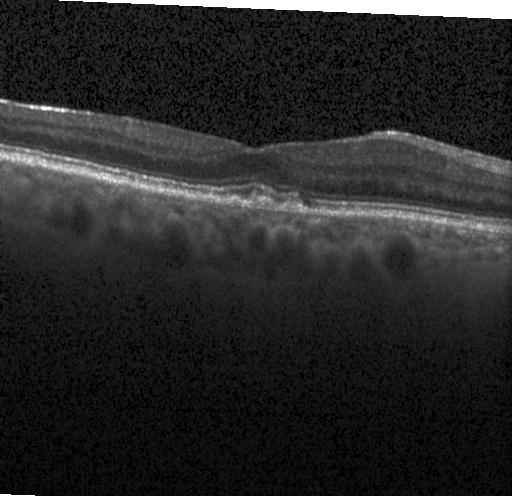

Through the macula · retinal OCT cross-section · SD-OCT.
Multiple drusen.